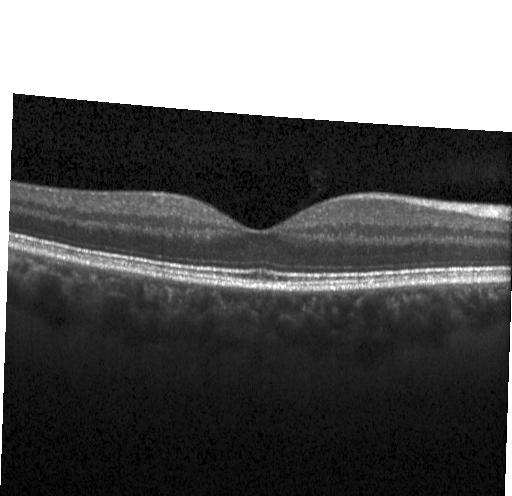

Dx: no evidence of choroidal neovascularization, diabetic macular edema, or drusen.